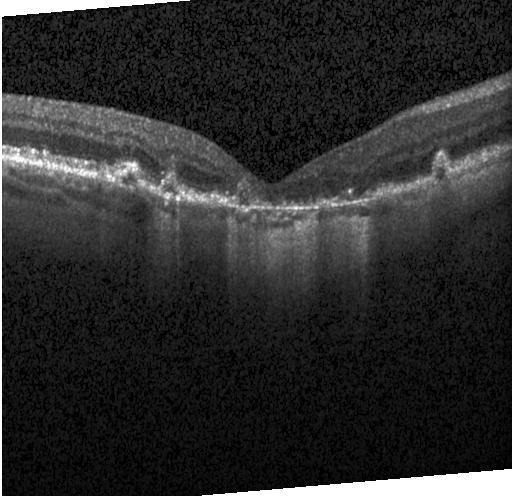
Optical coherence tomography B-scan; centered on the fovea; spectral-domain OCT; instrument: Heidelberg Spectralis. OCT finding: choroidal neovascularization.